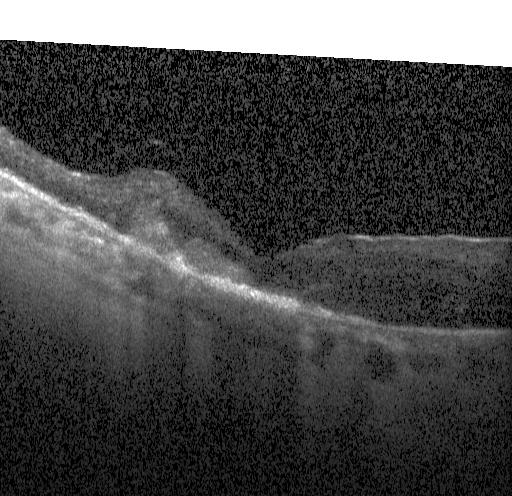

Diagnosis: a choroidal neovascular membrane.